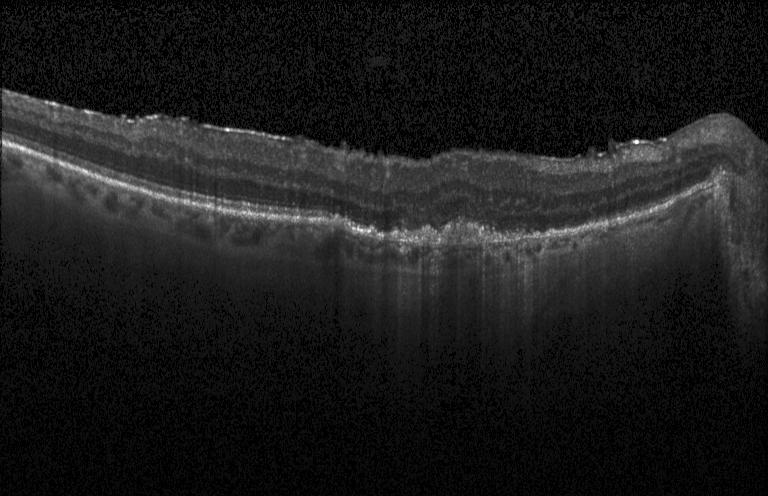

Optical coherence tomography scan
Macular OCT: a choroidal neovascular membrane.